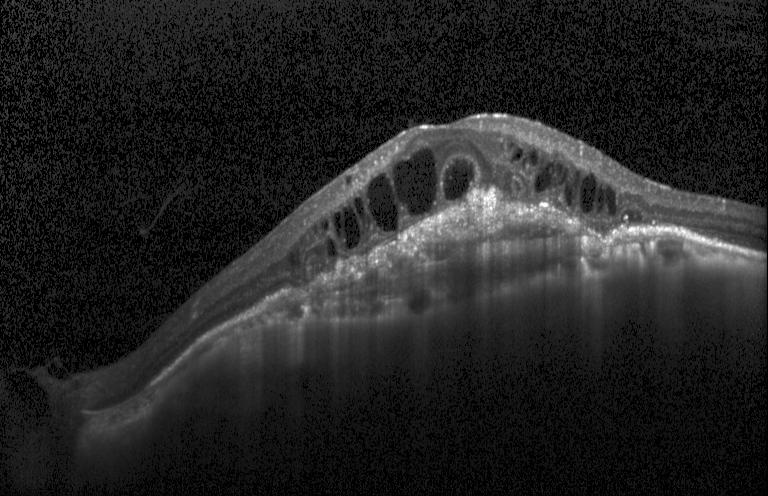 Fovea-centered, Heidelberg Spectralis, OCT line scan, SD-OCT. Dx: choroidal neovascularization.